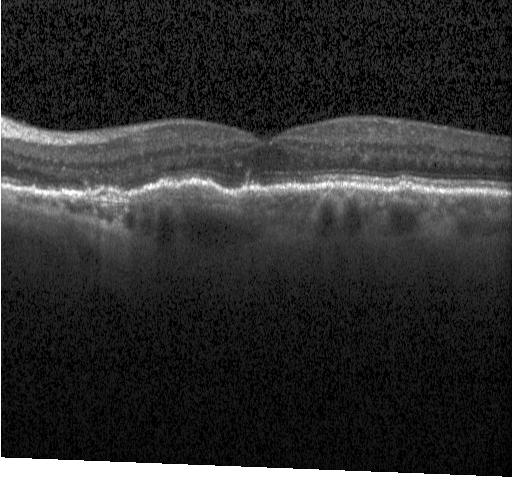

Heidelberg Spectralis OCT system, OCT line scan, macular scan, SD-OCT. The scan shows a choroidal neovascular membrane.